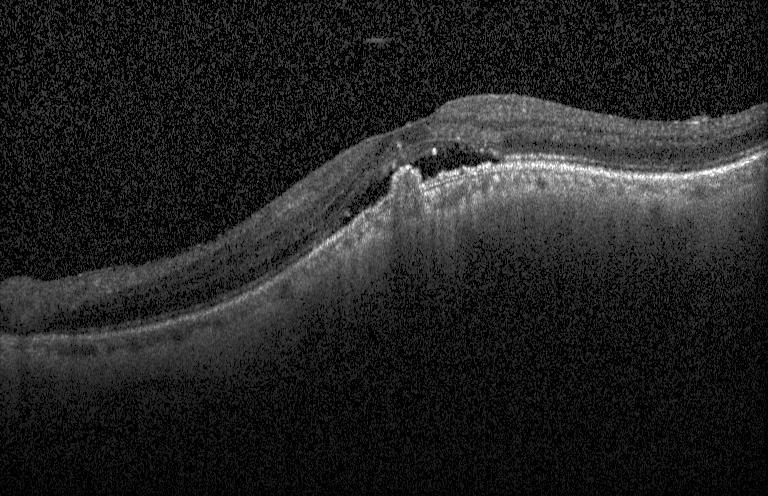 This B-scan demonstrates choroidal neovascularization.